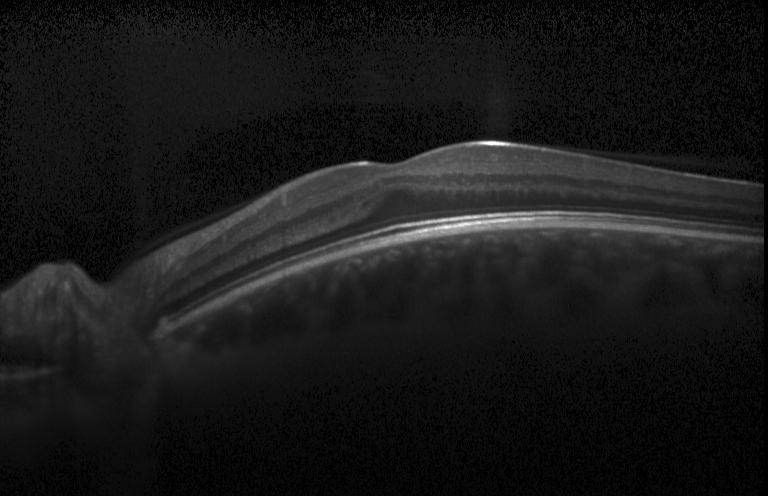 Finding: neither choroidal neovascularization, diabetic macular edema, nor drusen.